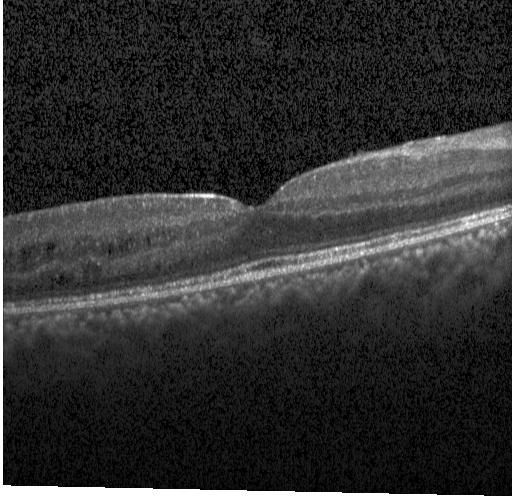 Retinal OCT B-scan, spectral-domain OCT
The scan shows diabetic macular edema (DME).